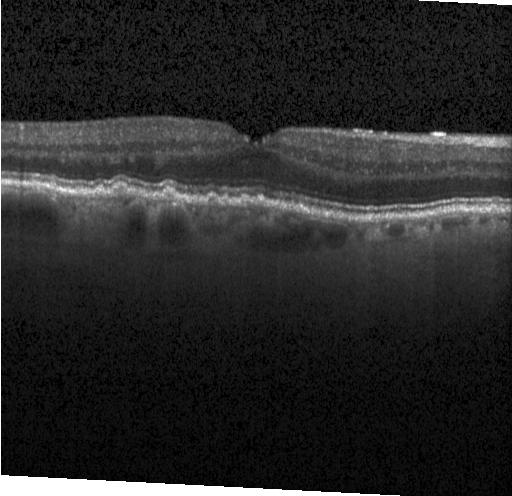 OCT B-scan showing drusen.